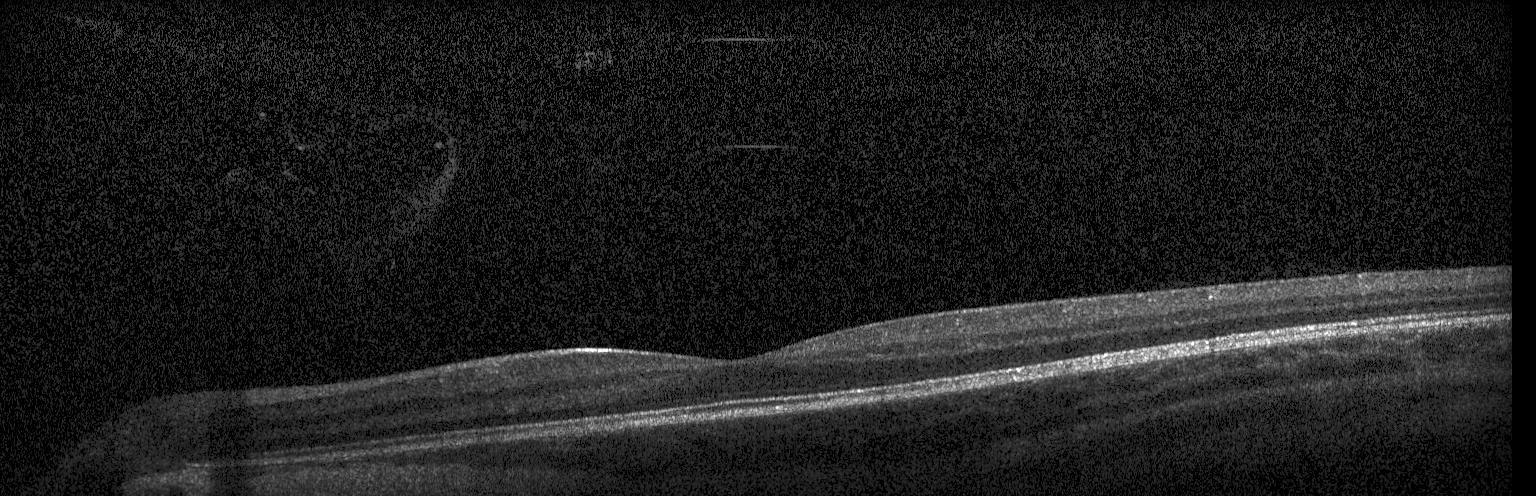
Fovea-centered. Retinal OCT B-scan
Assessment: no evidence of CNV, DME, or drusen.